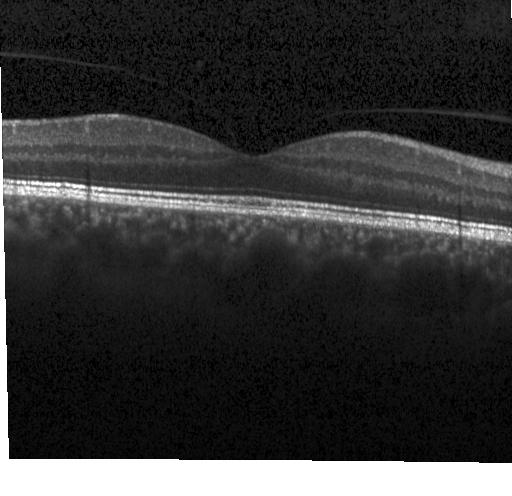 Optical coherence tomography B-scan — Diagnosis: no choroidal neovascularization, diabetic macular edema, or drusen.